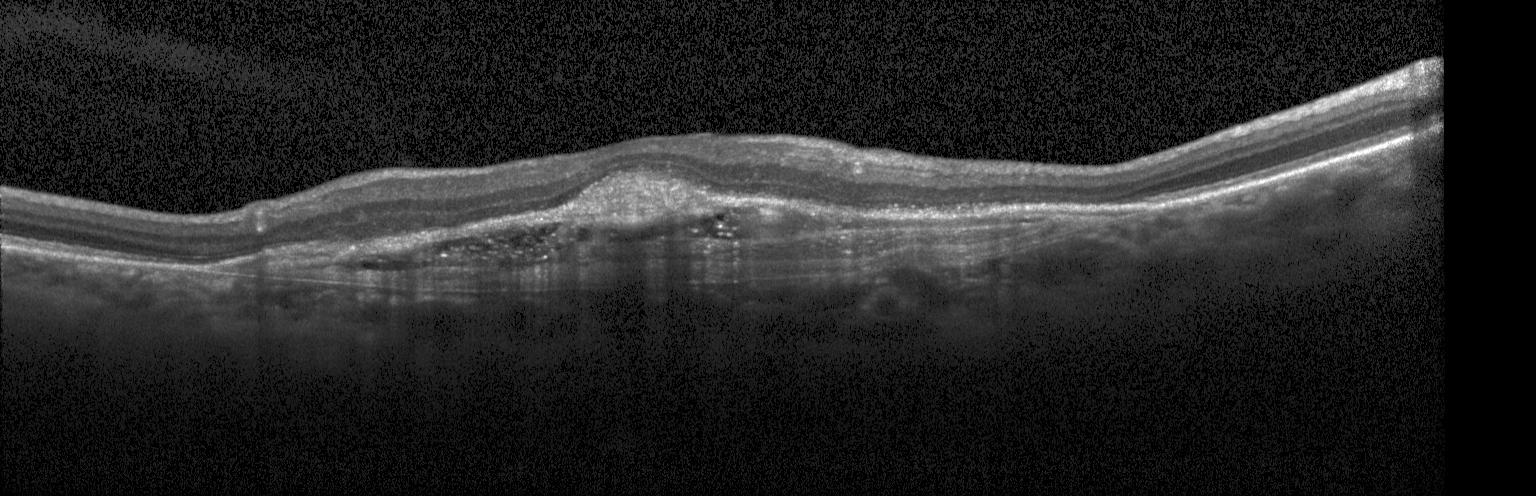 Optical coherence tomography B-scan — Assessment: choroidal neovascularization.